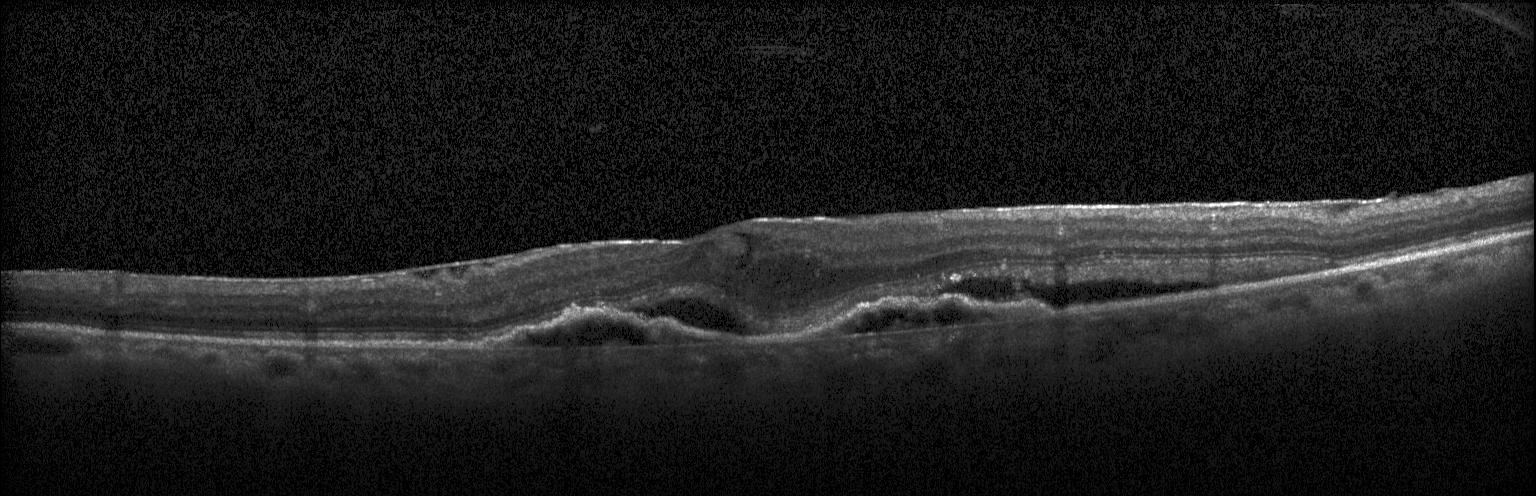

Impression: a choroidal neovascular membrane.